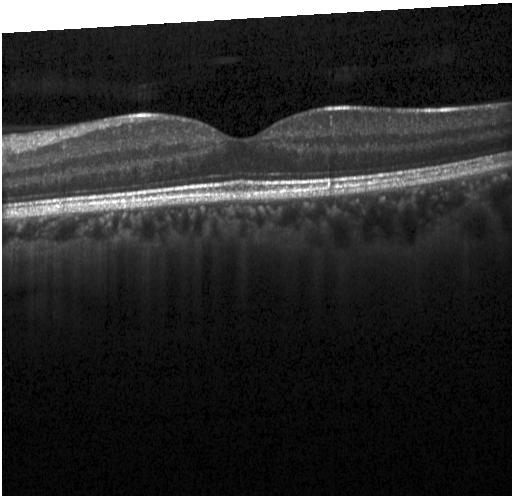

Fovea-centered, acquired on a Heidelberg Spectralis, SD-OCT, OCT B-scan — Dx: no evidence of CNV, DME, or drusen.